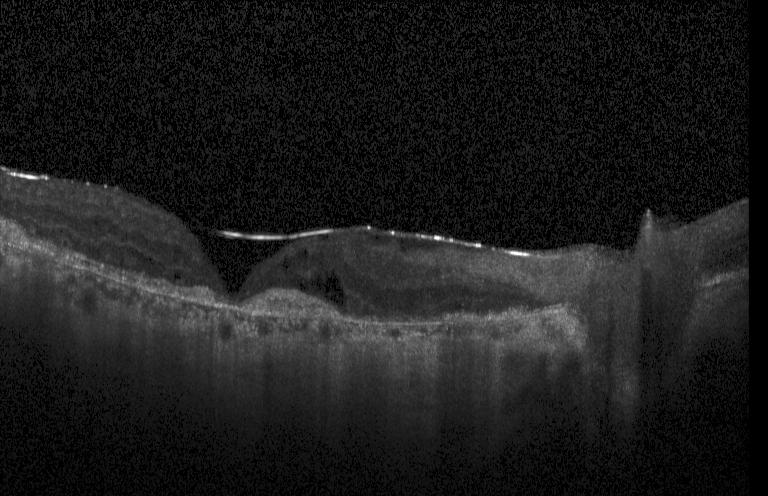
Spectral-domain OCT, retinal OCT B-scan, horizontal scan through the fovea
Diagnosis: a choroidal neovascular membrane.